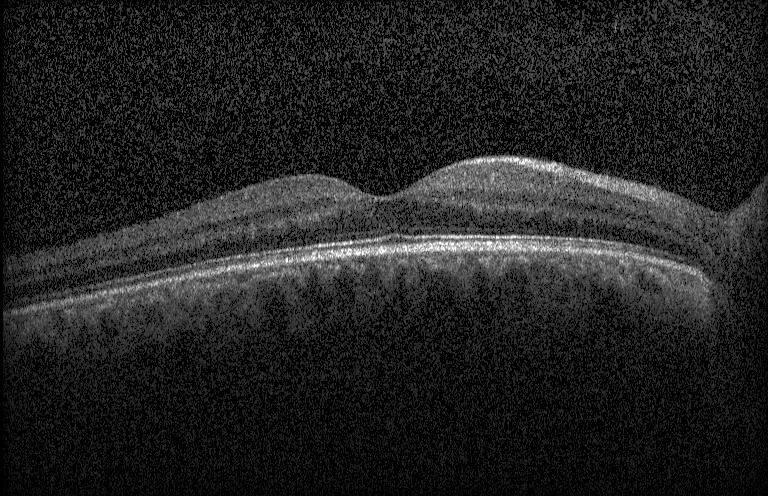
Spectral-domain OCT B-scan: no choroidal neovascularization, no diabetic macular edema, and no drusen.